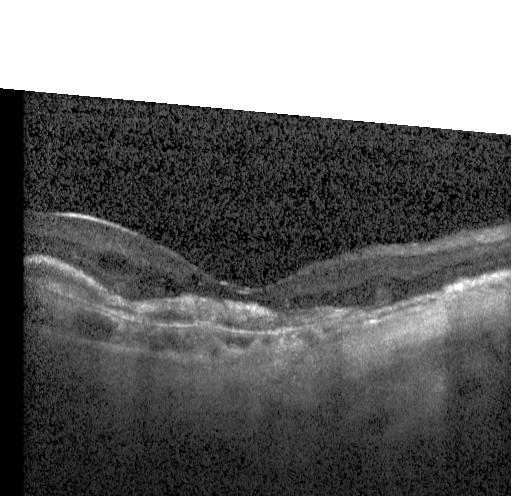

OCT line scan
Finding: a choroidal neovascular membrane.